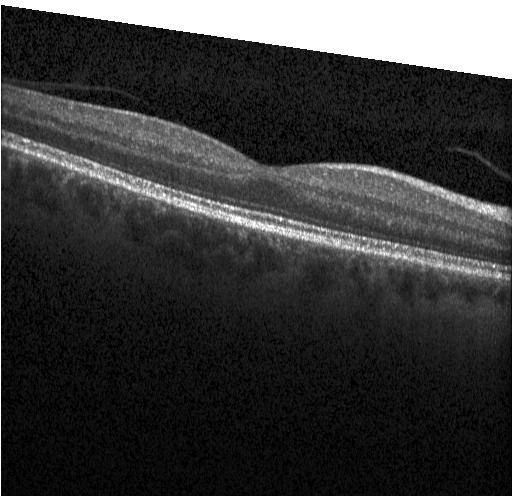

Optical coherence tomography scan, horizontal scan through the fovea, spectral-domain OCT, acquired on a Heidelberg Spectralis
Dx: no evidence of CNV, DME, or drusen.